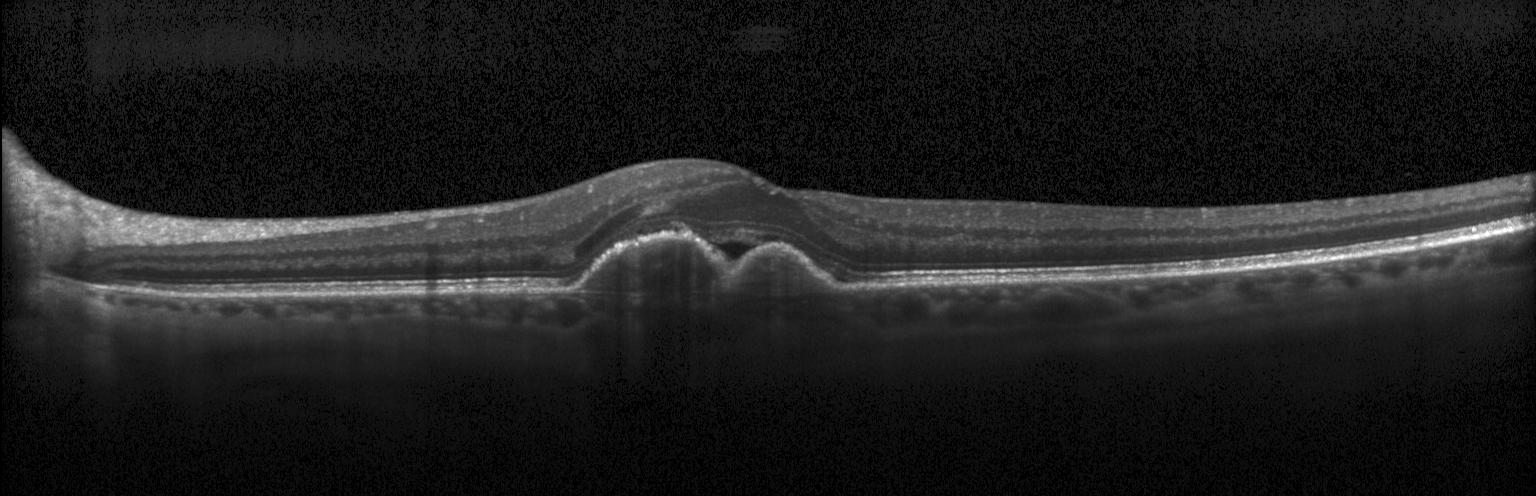

Dx: choroidal neovascularization.